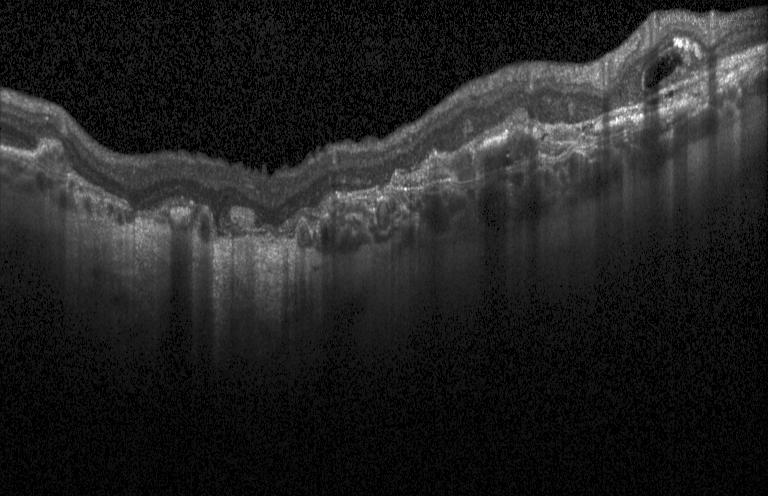

Optical coherence tomography scan. Acquired on a Heidelberg Spectralis — Assessment: a choroidal neovascular membrane.